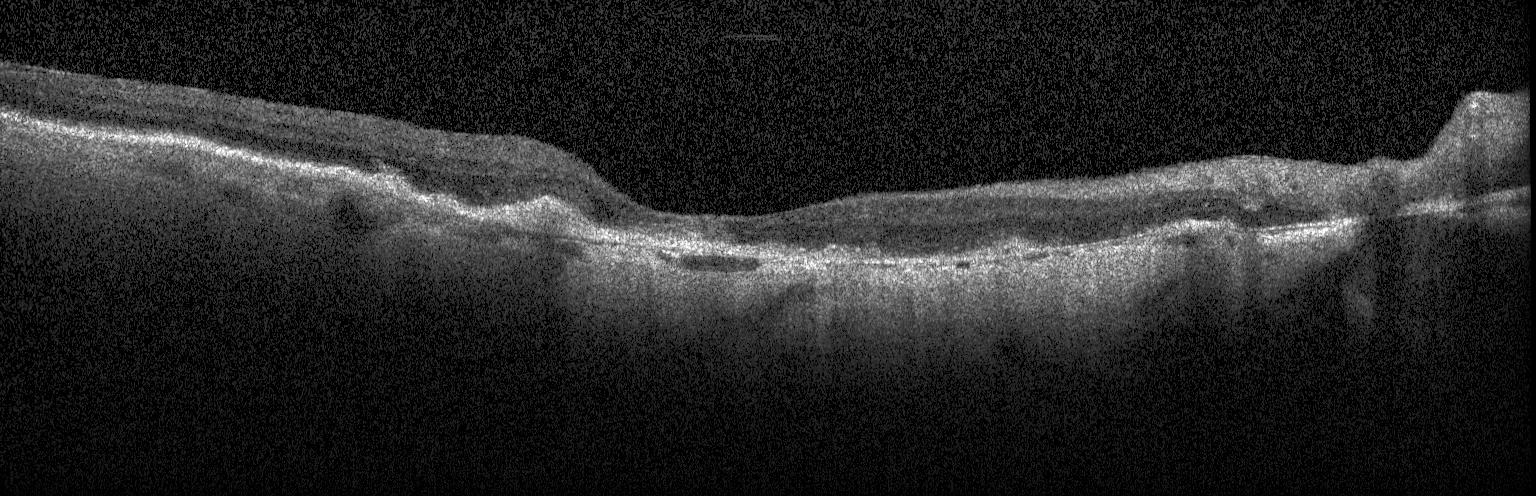
This B-scan demonstrates choroidal neovascularization (CNV).